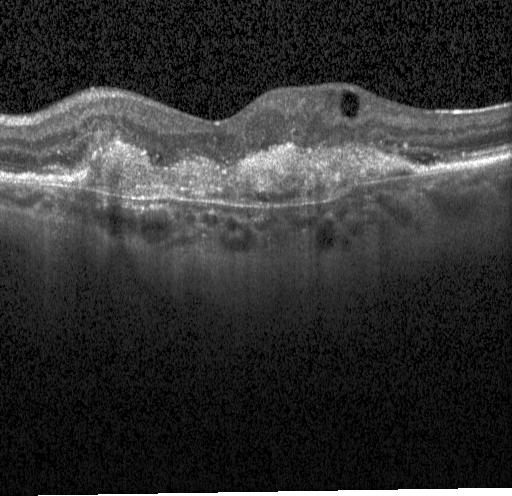

OCT B-scan; through the macula.
Impression: choroidal neovascularization.